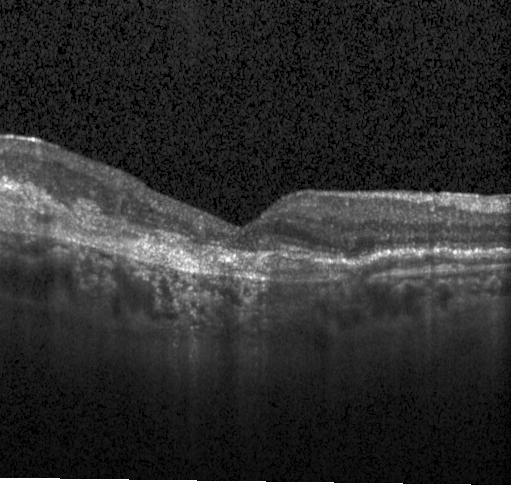
OCT finding: CNV.